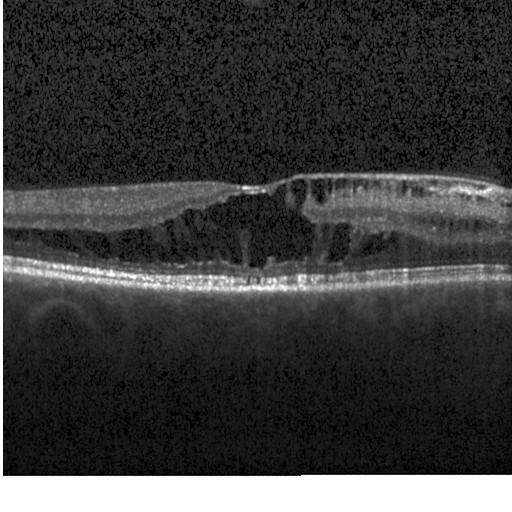
Diagnosis: diabetic macular edema.